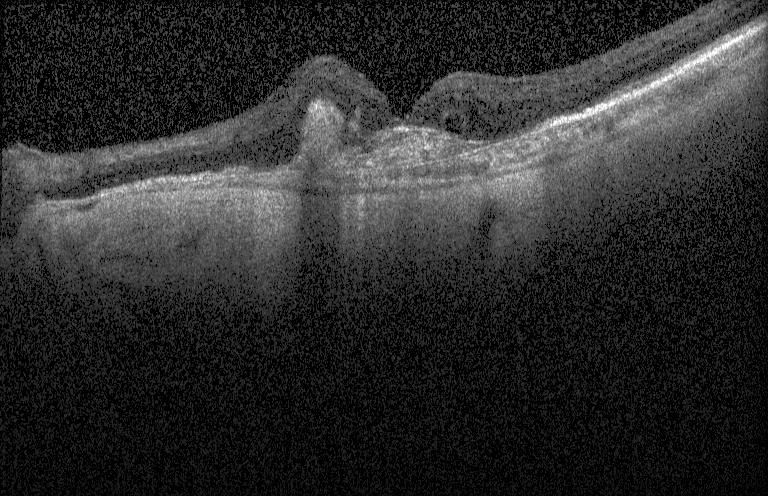
OCT scan showing choroidal neovascularization.